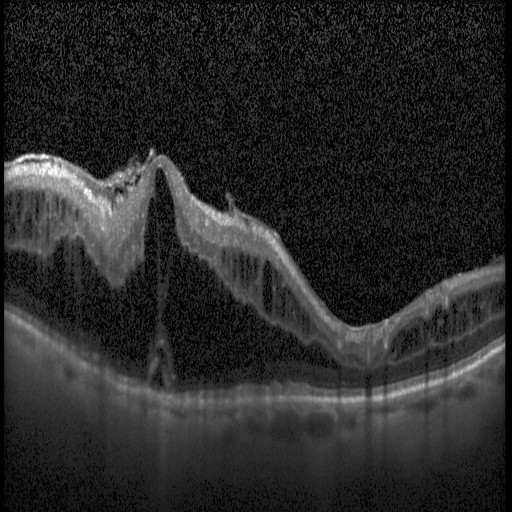
Retinal OCT cross-section · Heidelberg Spectralis.
Impression: DME.